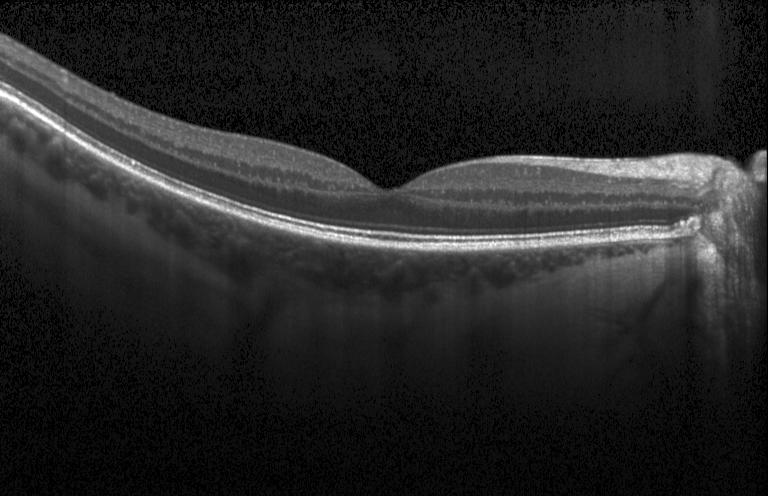

Retinal OCT B-scan · SD-OCT · Heidelberg Spectralis · through the macula — Macular OCT: no choroidal neovascularization, no diabetic macular edema, and no drusen.